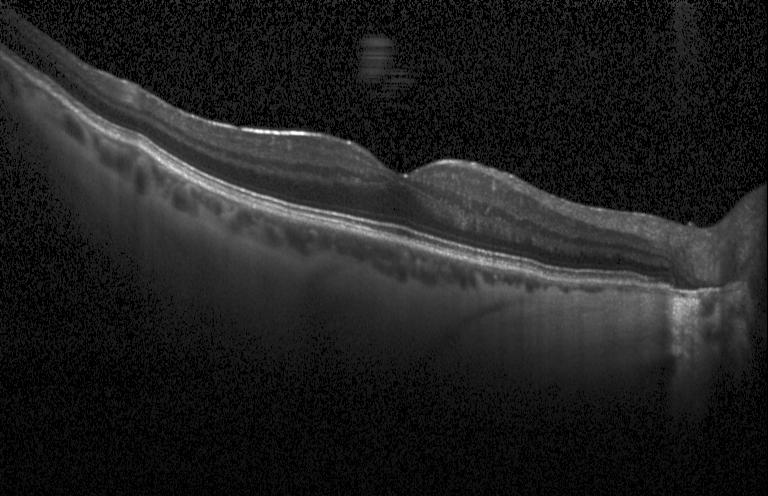 Spectral-domain optical coherence tomography; OCT line scan; Heidelberg Spectralis OCT system — The scan shows no choroidal neovascularization, no diabetic macular edema, and no drusen.